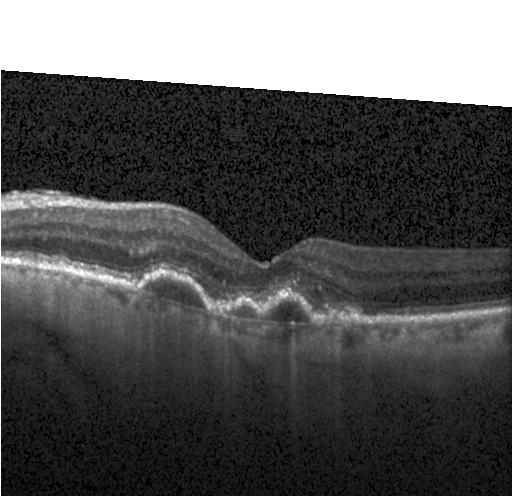

Instrument: Heidelberg Spectralis; spectral-domain optical coherence tomography; horizontal scan through the fovea; optical coherence tomography scan. Finding: a choroidal neovascular membrane.